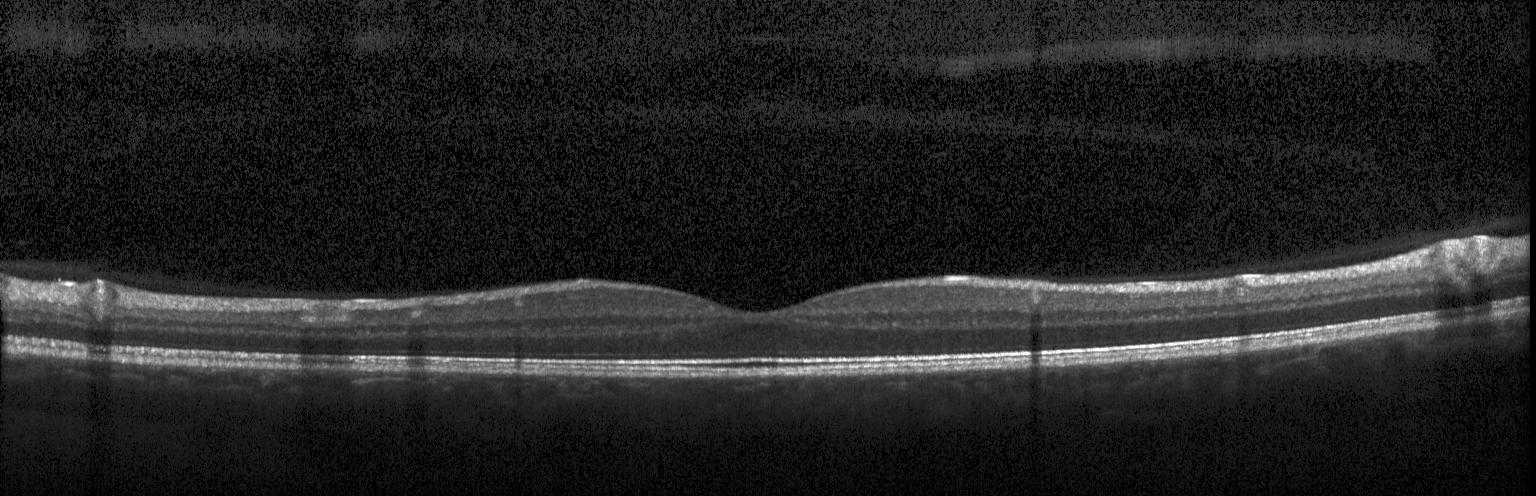

OCT line scan
The scan shows no choroidal neovascularization, no diabetic macular edema, and no drusen.